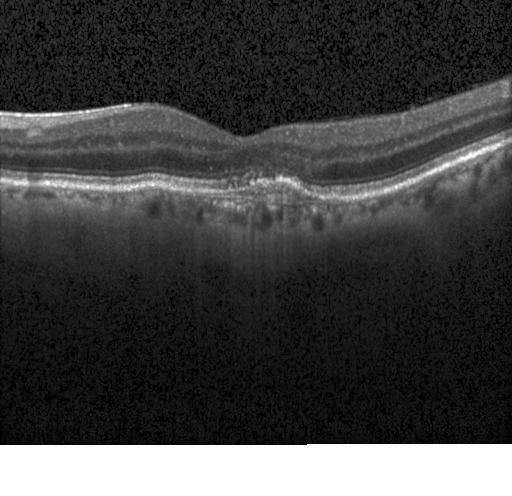

Assessment: CNV.